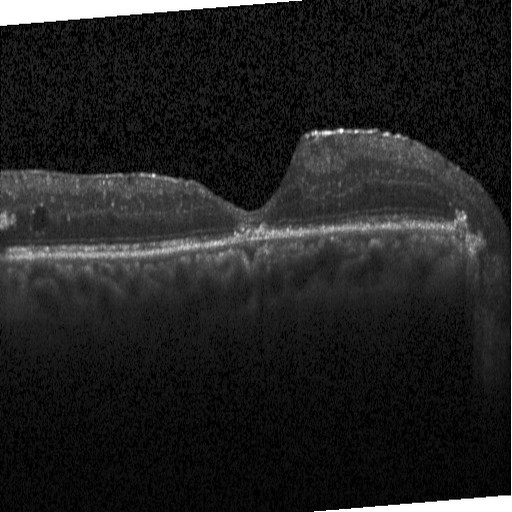 OCT scan showing diabetic macular edema.